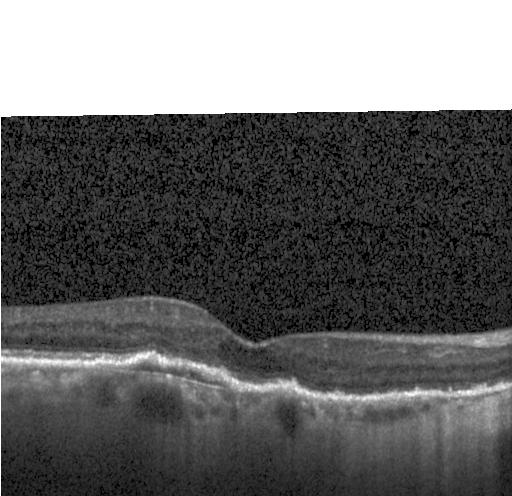 Optical coherence tomography scan; Heidelberg Spectralis. This B-scan demonstrates a choroidal neovascular membrane.